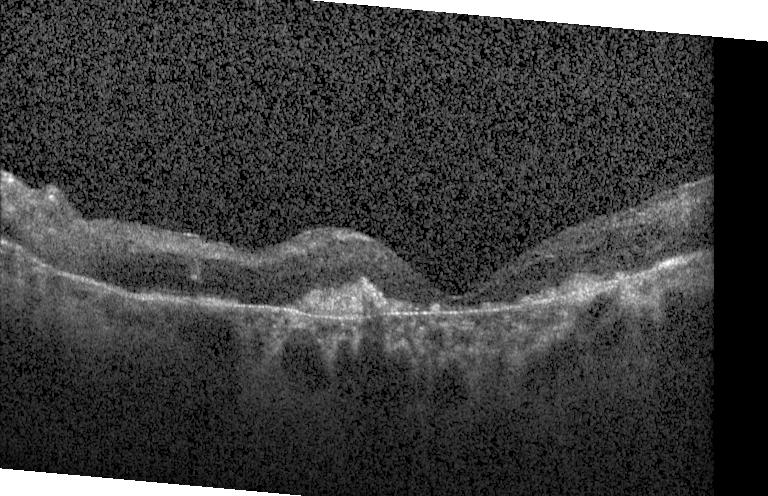 Instrument: Heidelberg Spectralis; retinal OCT B-scan; spectral-domain optical coherence tomography. Impression: choroidal neovascularization (CNV).